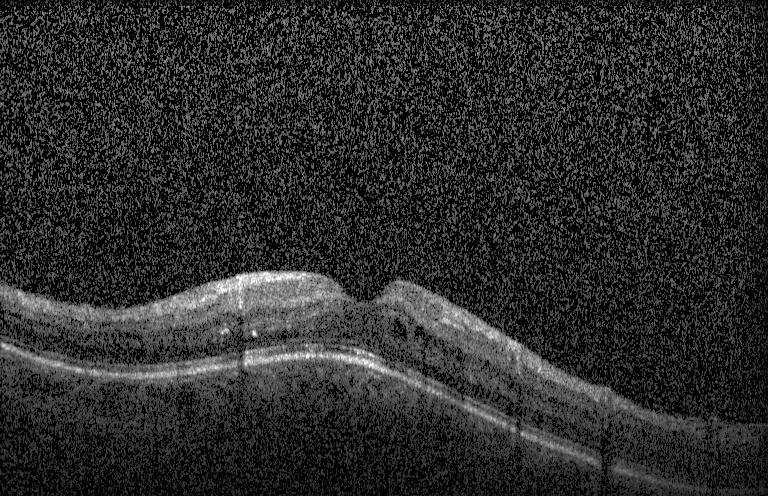

Horizontal scan through the fovea; optical coherence tomography scan; instrument: Heidelberg Spectralis — Diagnosis: DME.